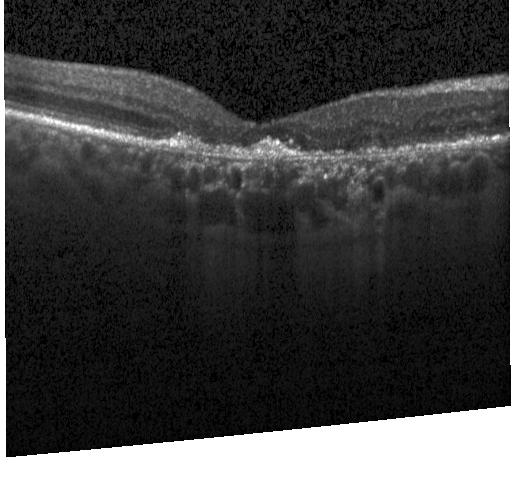

Centered on the fovea. SD-OCT. Heidelberg Spectralis. Optical coherence tomography B-scan.
Finding: choroidal neovascularization (CNV).